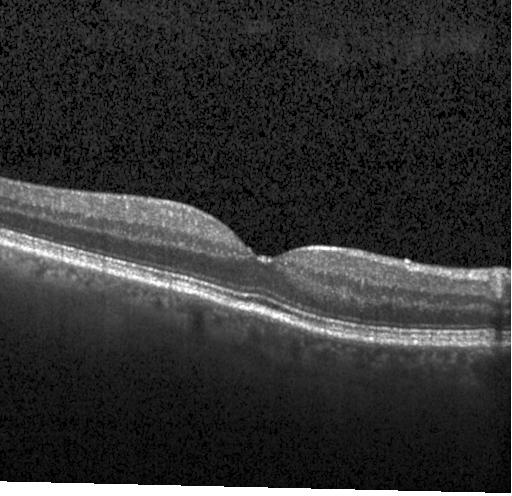

Heidelberg Spectralis, OCT line scan.
Macular OCT: no choroidal neovascularization, diabetic macular edema, or drusen.